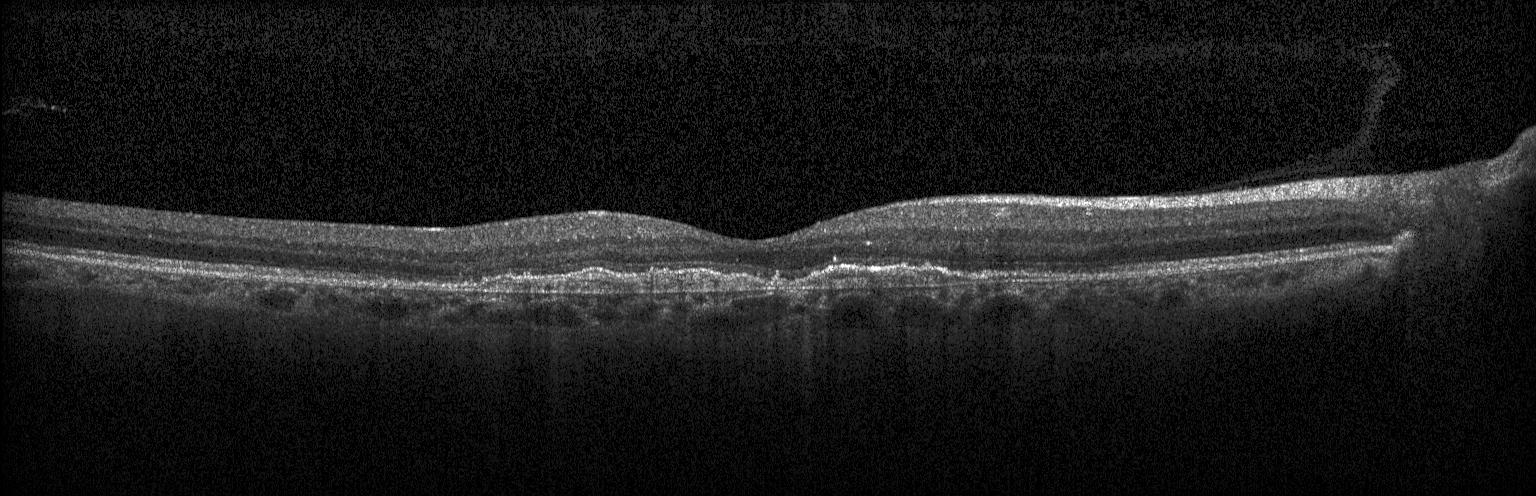

Retinal OCT cross-section.
This B-scan demonstrates a choroidal neovascular membrane.